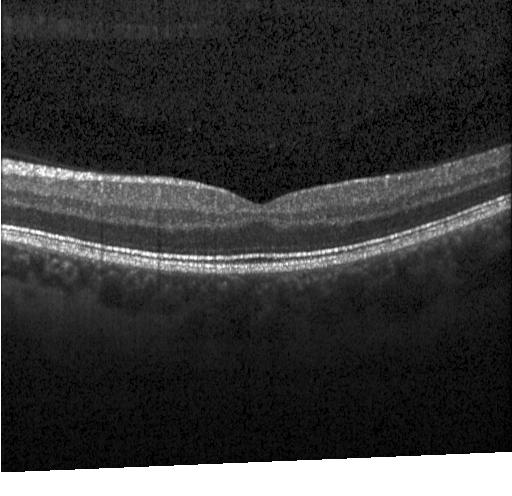

Assessment: neither choroidal neovascularization, diabetic macular edema, nor drusen.